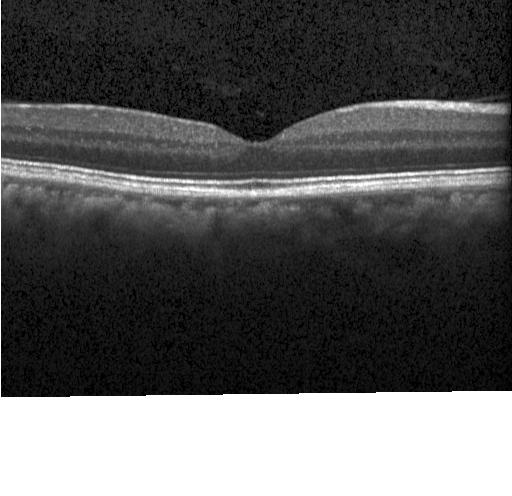 Spectral-domain OCT. Horizontal scan through the fovea. OCT line scan.
Dx: no evidence of choroidal neovascularization, diabetic macular edema, or drusen.